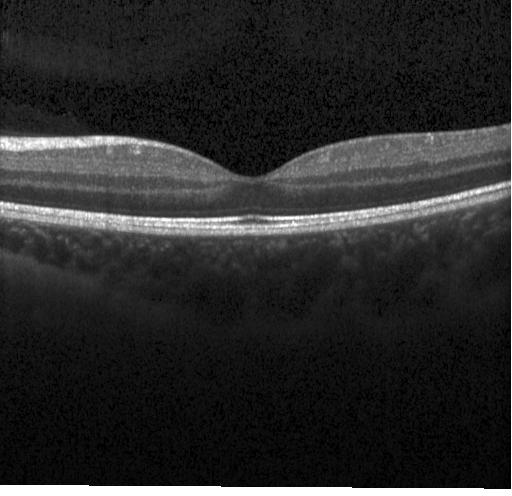 Spectral-domain OCT. Instrument: Heidelberg Spectralis. Optical coherence tomography B-scan. Macular scan — Impression: no choroidal neovascularization, no diabetic macular edema, and no drusen.